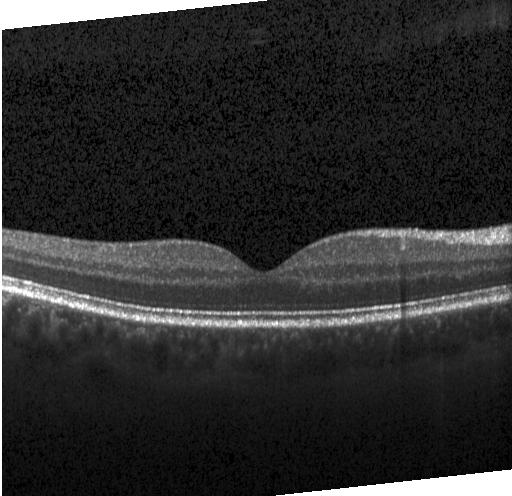
Spectral-domain OCT B-scan: no CNV, no DME, and no drusen.